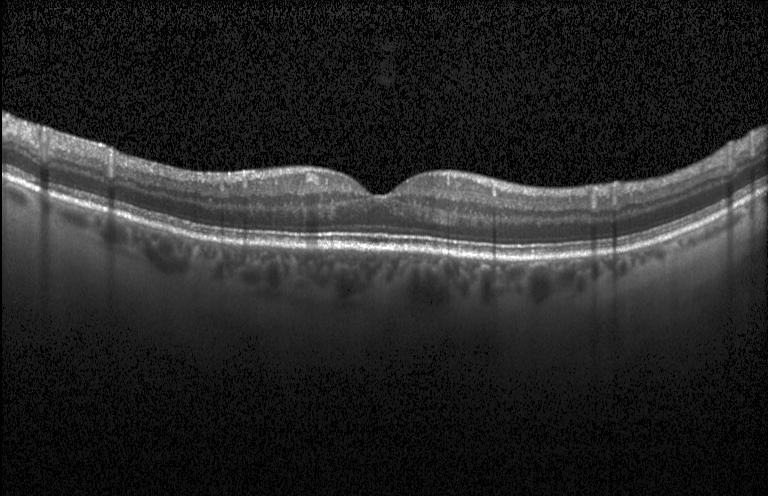

Retinal OCT B-scan.
Diagnosis: no choroidal neovascularization, no diabetic macular edema, and no drusen.